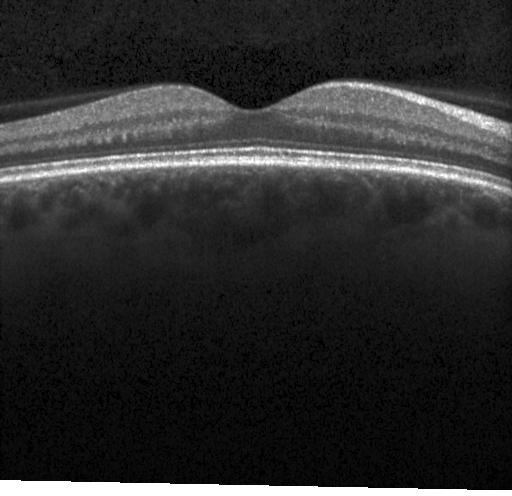

OCT B-scan. Macular scan.
No CNV, no DME, and no drusen.